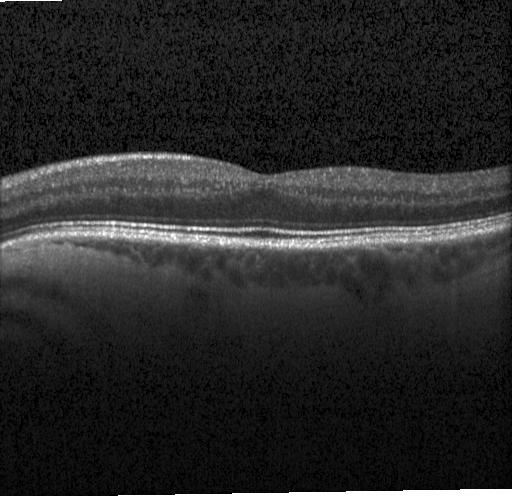

Retinal OCT B-scan — Finding: no choroidal neovascularization, diabetic macular edema, or drusen.